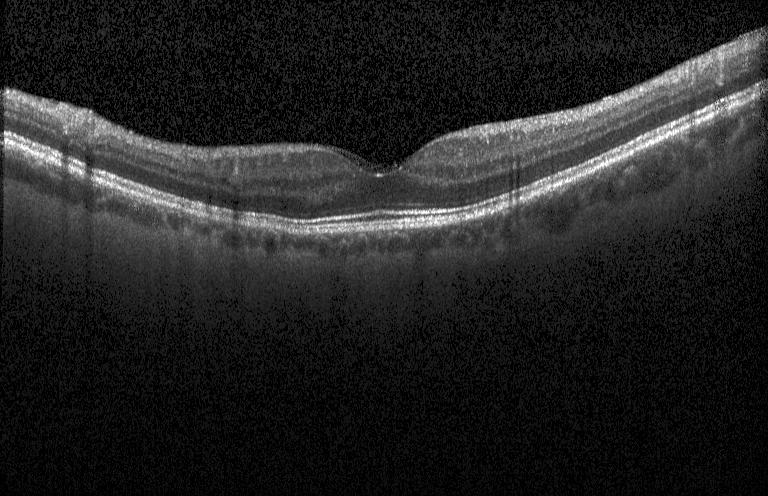

Retinal OCT cross-section.
This B-scan demonstrates no choroidal neovascularization, no diabetic macular edema, and no drusen.